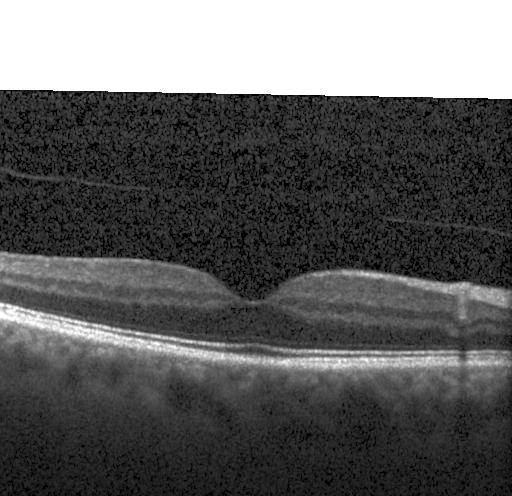 Finding: no evidence of choroidal neovascularization, diabetic macular edema, or drusen.